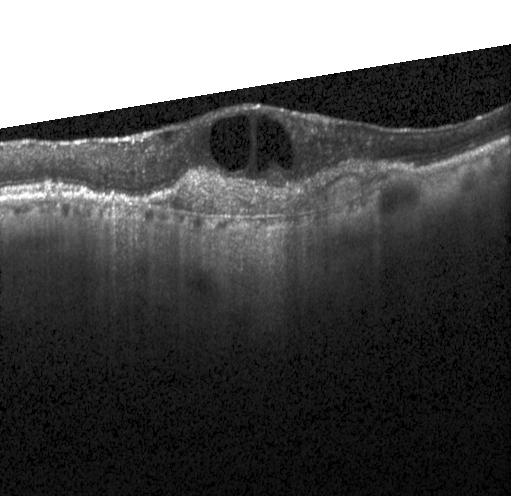
Spectral-domain OCT B-scan: CNV.